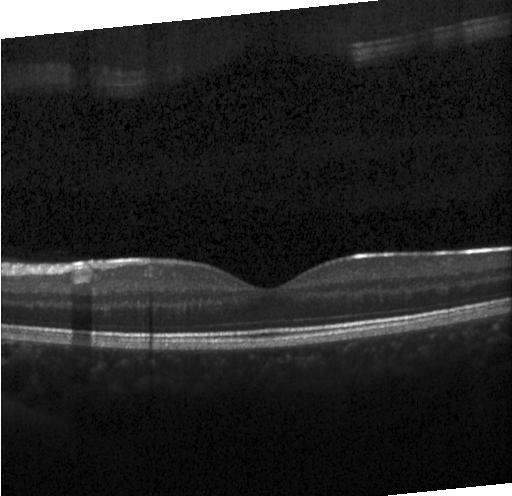

OCT scan showing neither choroidal neovascularization, diabetic macular edema, nor drusen.